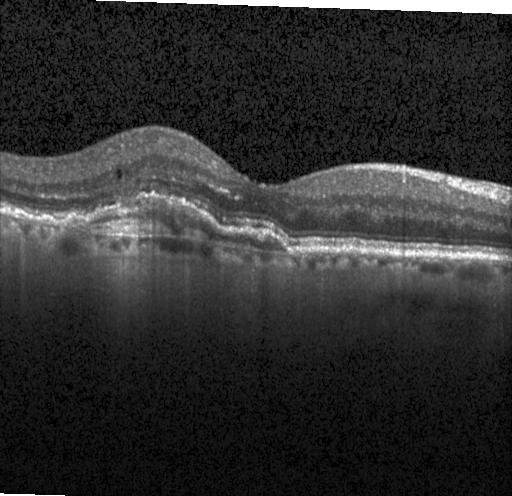
Macular OCT: a choroidal neovascular membrane.